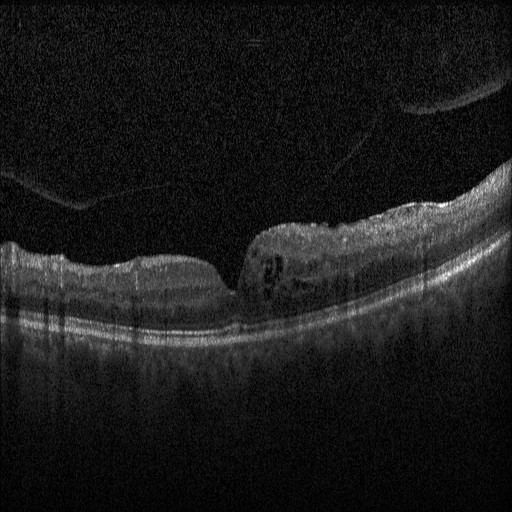

OCT B-scan showing diabetic macular edema (DME).